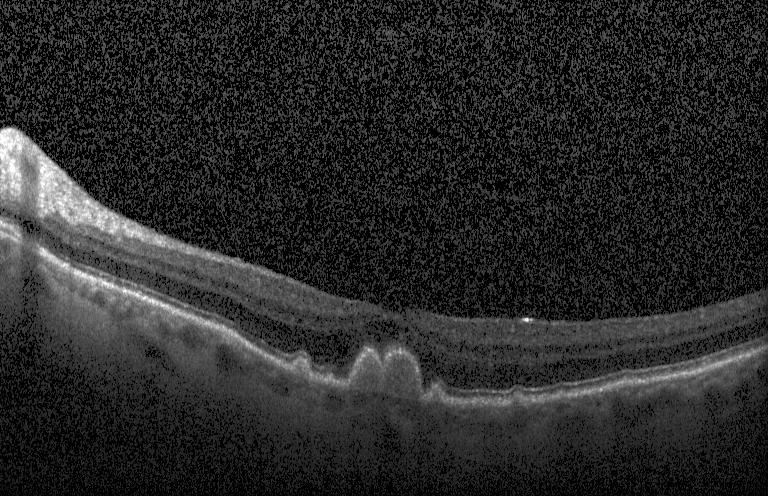 Finding: multiple drusen.